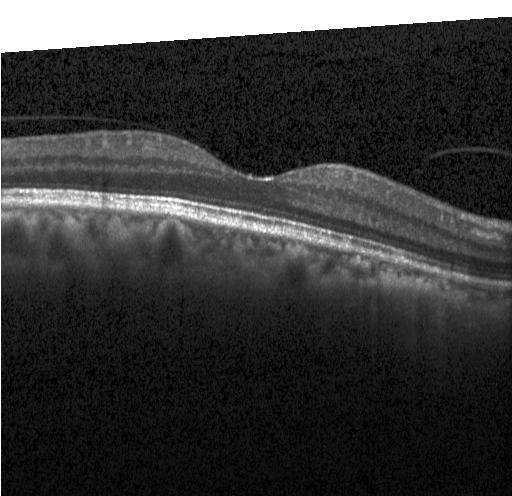

Horizontal scan through the fovea, OCT line scan, spectral-domain OCT, instrument: Heidelberg Spectralis.
OCT finding: no choroidal neovascularization, diabetic macular edema, or drusen.